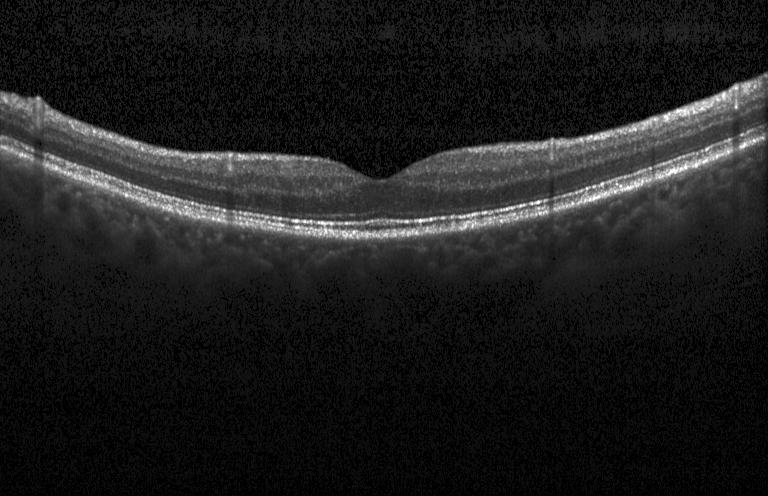
OCT line scan, centered on the fovea.
OCT finding: no evidence of choroidal neovascularization, diabetic macular edema, or drusen.